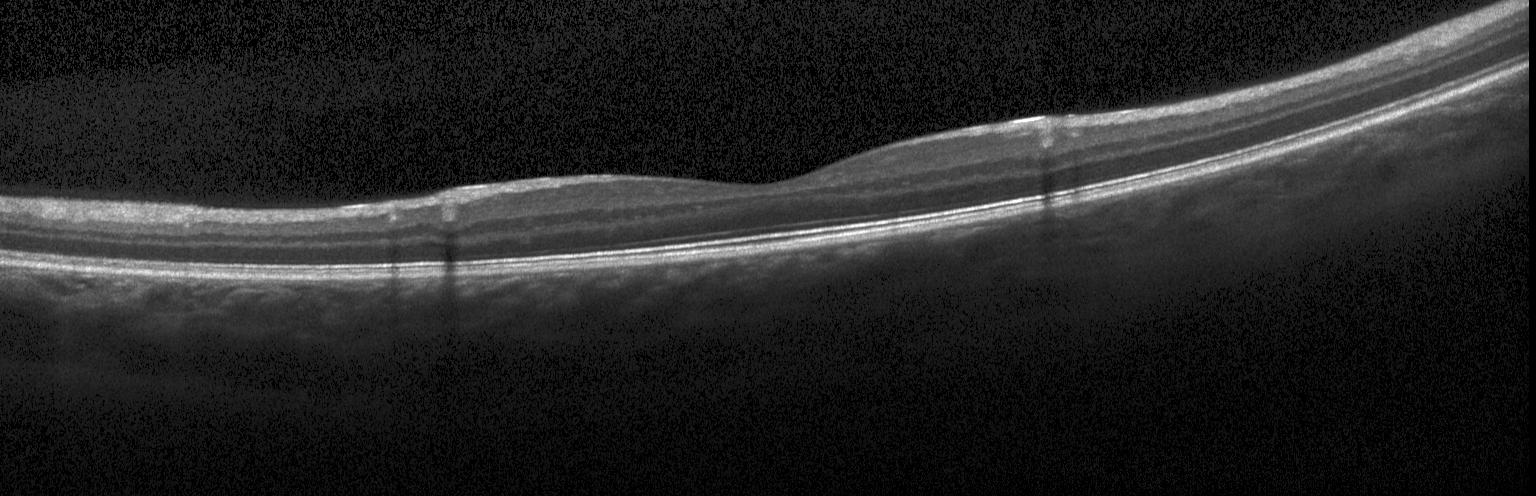
Through the macula. SD-OCT. Optical coherence tomography scan. OCT finding: no choroidal neovascularization, diabetic macular edema, or drusen.